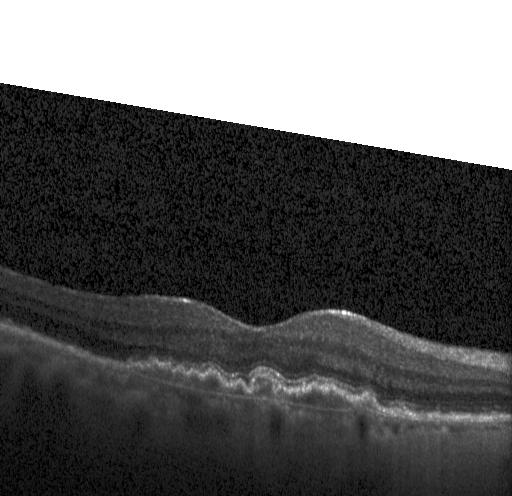

Spectral-domain OCT B-scan: choroidal neovascularization.